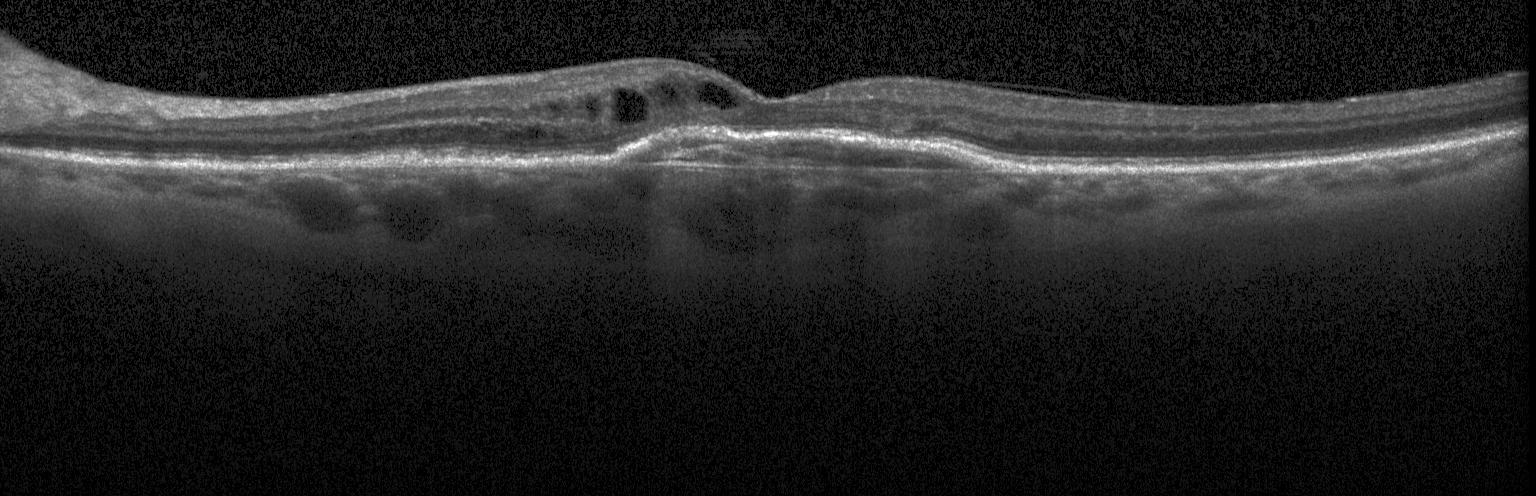

Spectral-domain OCT B-scan: a choroidal neovascular membrane.